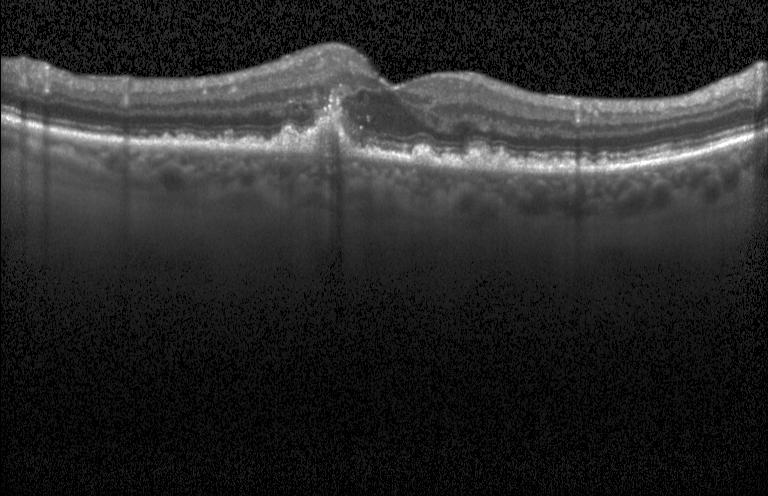

Acquired on a Heidelberg Spectralis; optical coherence tomography scan — Macular OCT: choroidal neovascularization.